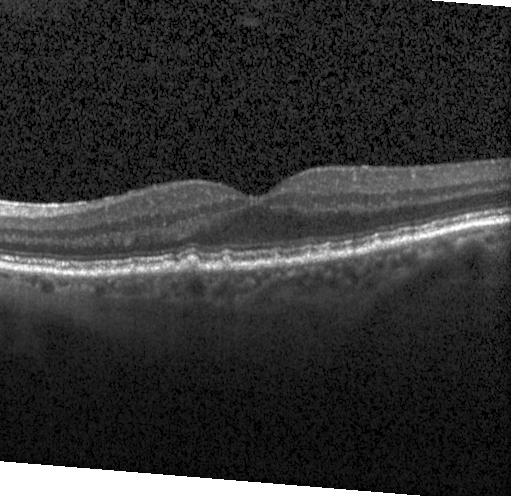
OCT B-scan, spectral-domain optical coherence tomography, through the macula. Diagnosis: drusen.